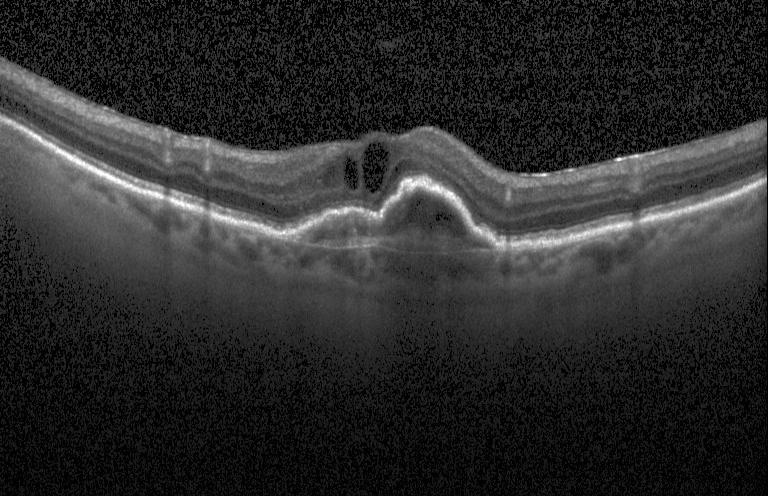
Horizontal scan through the fovea, instrument: Heidelberg Spectralis, optical coherence tomography scan, spectral-domain optical coherence tomography. Diagnosis: choroidal neovascularization.